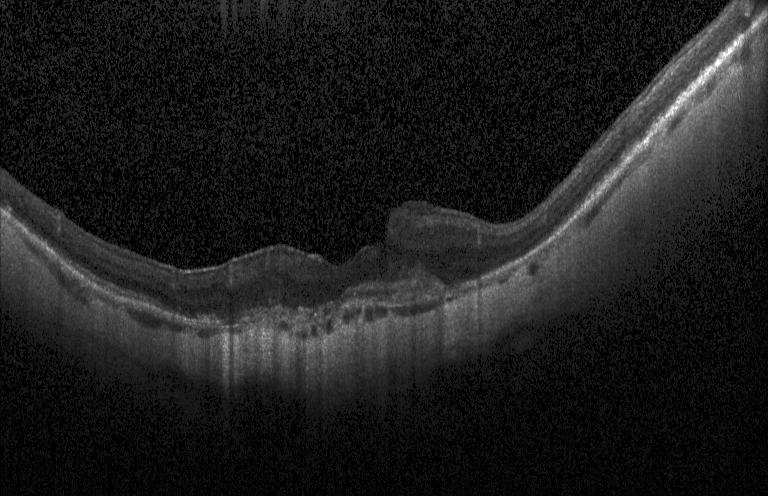
OCT B-scan, instrument: Heidelberg Spectralis, horizontal scan through the fovea. The scan shows a choroidal neovascular membrane.